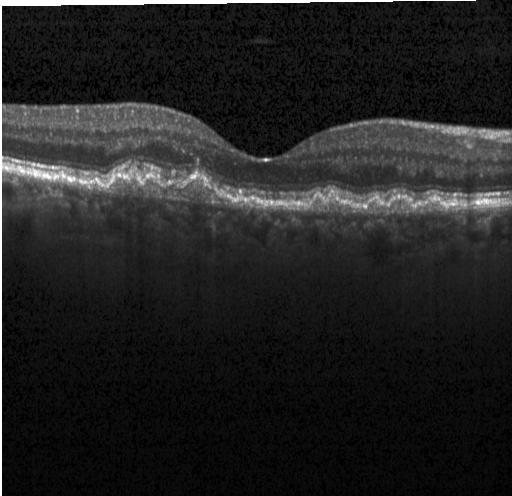
Dx: choroidal neovascularization.